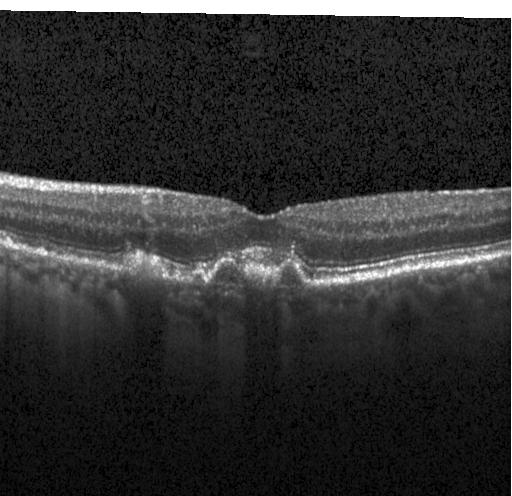
Macular OCT demonstrating choroidal neovascularization (CNV).